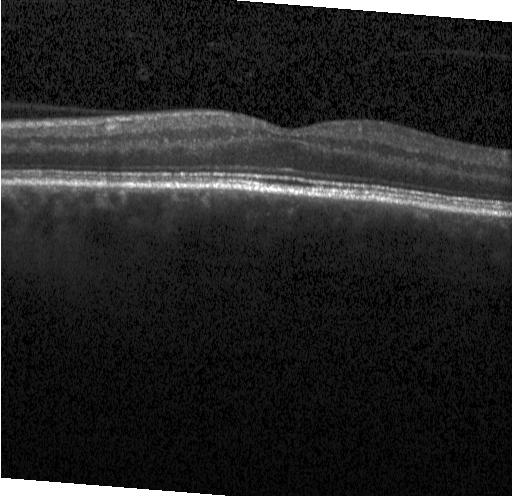

Neither choroidal neovascularization, diabetic macular edema, nor drusen.